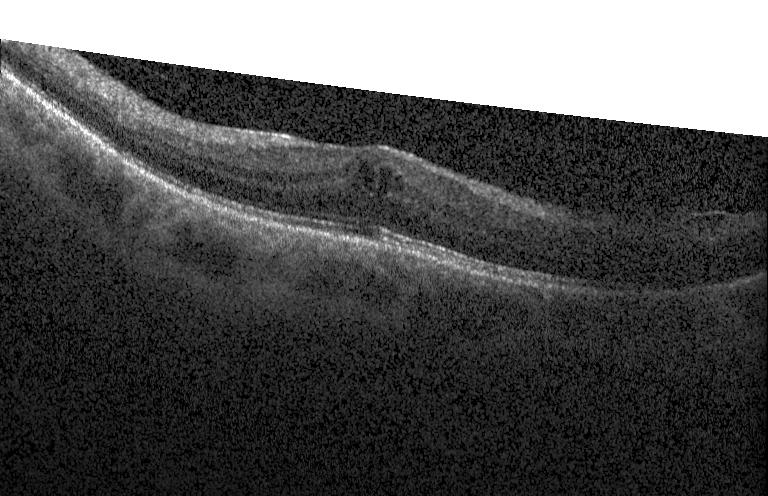

Impression: DME.